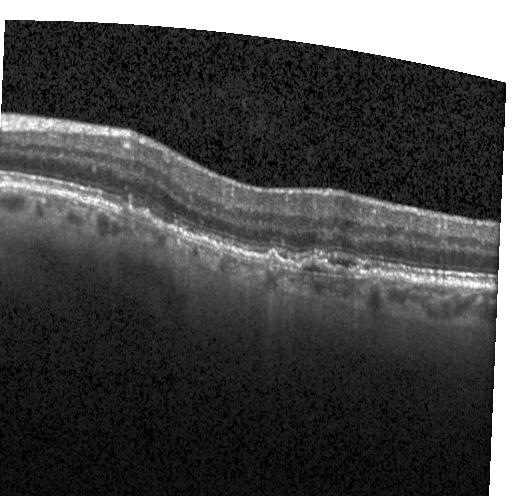 Impression: a choroidal neovascular membrane.